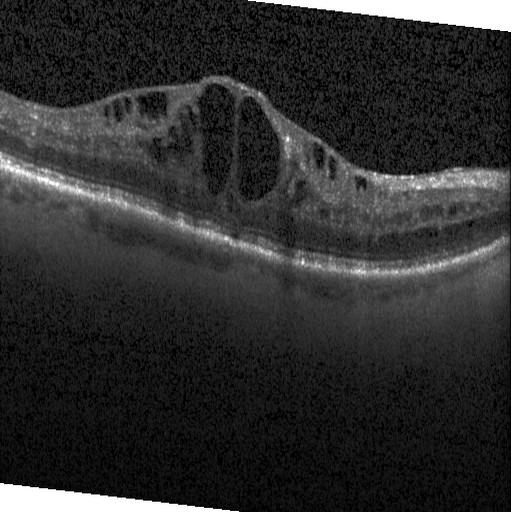
Macular scan. Heidelberg Spectralis. Spectral-domain optical coherence tomography. Retinal OCT cross-section
Assessment: diabetic macular edema (DME).